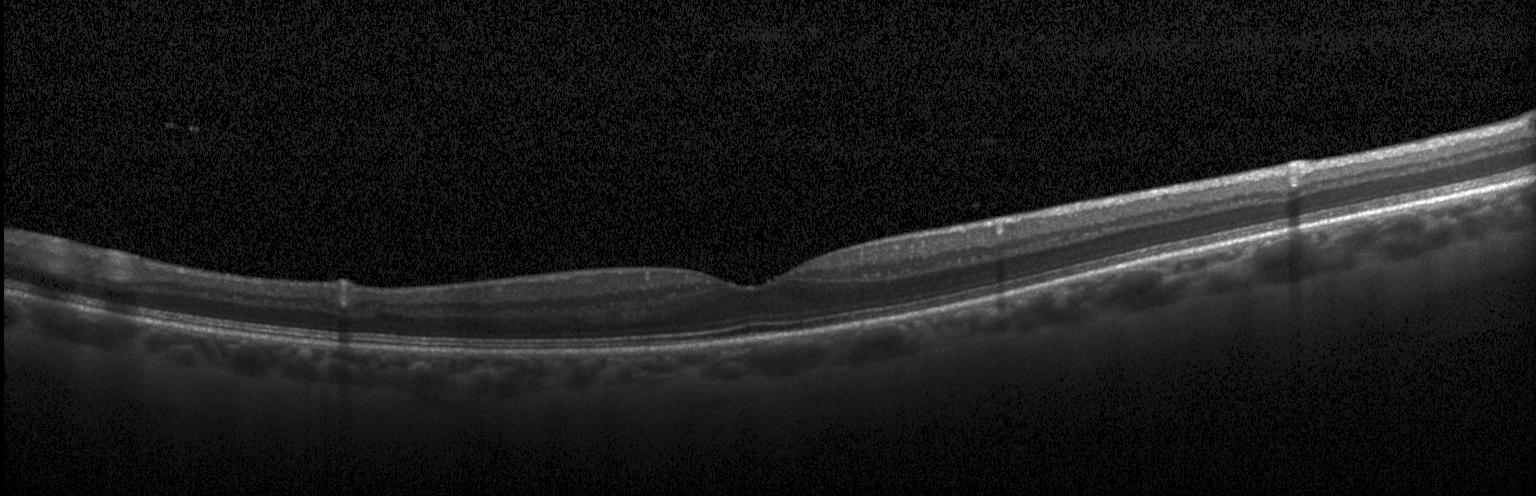
Macular scan. Retinal OCT B-scan. Spectral-domain OCT
Diagnosis: no CNV, no DME, and no drusen.